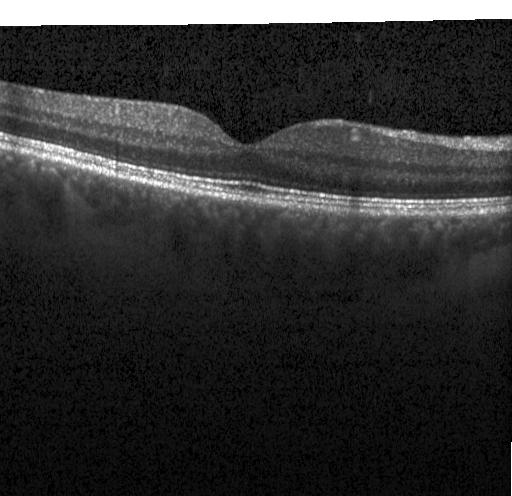
Finding: no choroidal neovascularization, no diabetic macular edema, and no drusen.